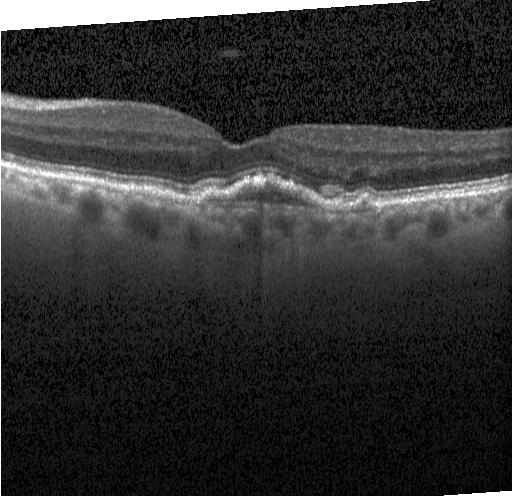 Impression: choroidal neovascularization.